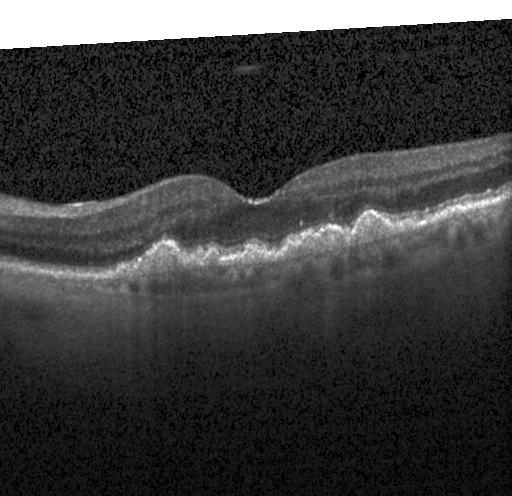

OCT line scan.
Finding: multiple drusen.